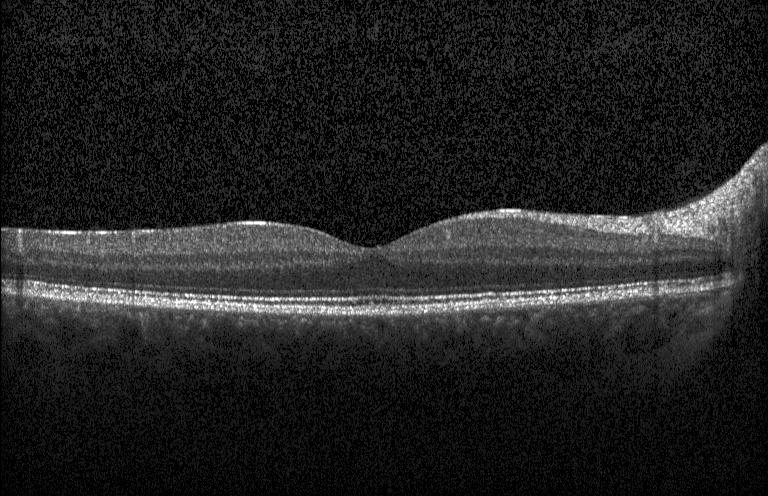 Macular scan. Optical coherence tomography B-scan — Dx: no evidence of CNV, DME, or drusen.